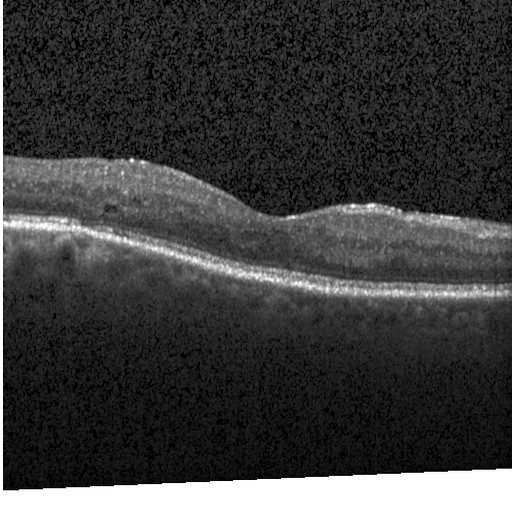 Retinal OCT cross-section showing diabetic macular edema.